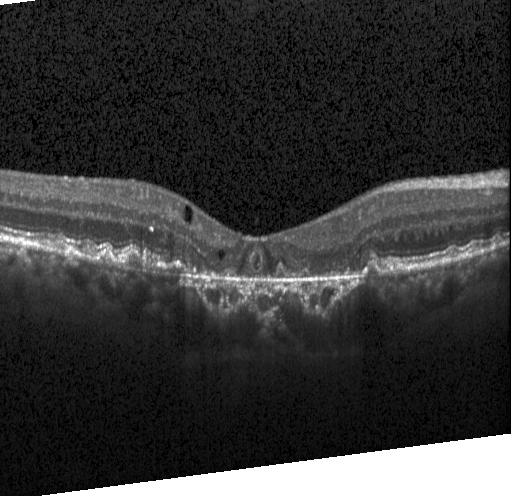
Diagnosis: choroidal neovascularization.